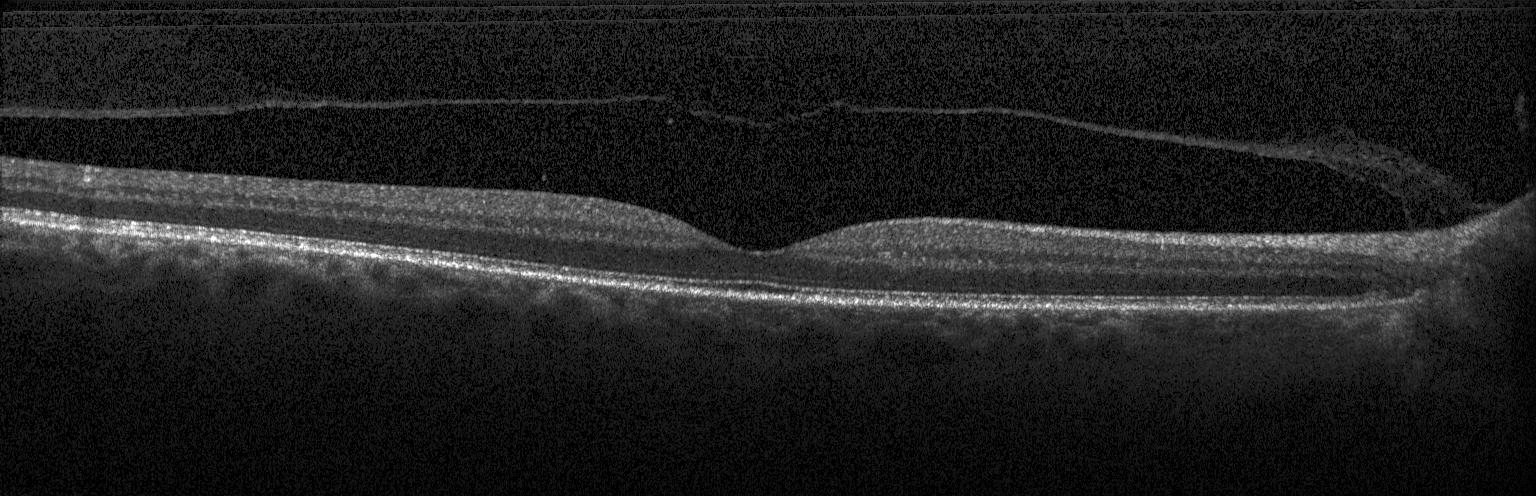
Impression: no CNV, no DME, and no drusen.